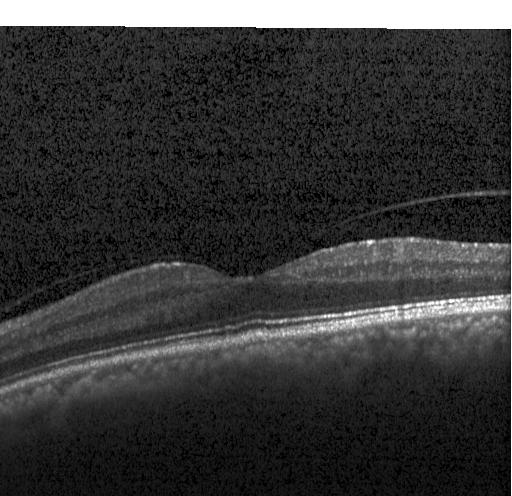 Diagnosis: neither CNV, DME, nor drusen.